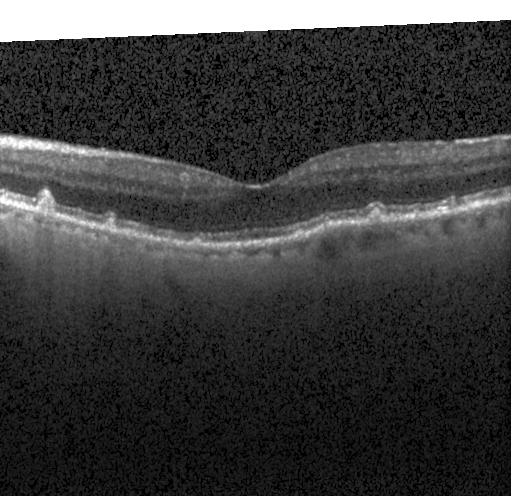

Macular OCT: multiple drusen.